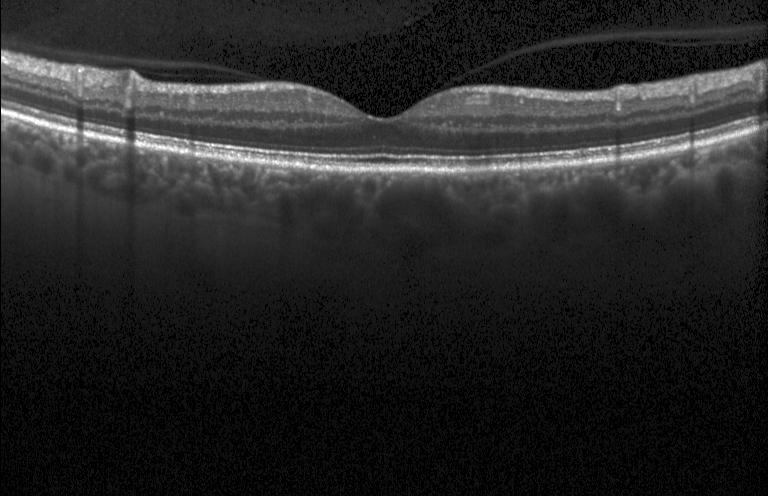 Retinal OCT cross-section. The scan shows neither choroidal neovascularization, diabetic macular edema, nor drusen.